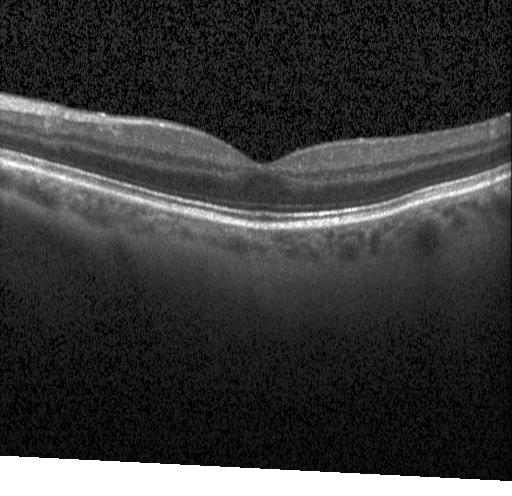

Horizontal scan through the fovea · retinal OCT cross-section.
OCT finding: no choroidal neovascularization, no diabetic macular edema, and no drusen.